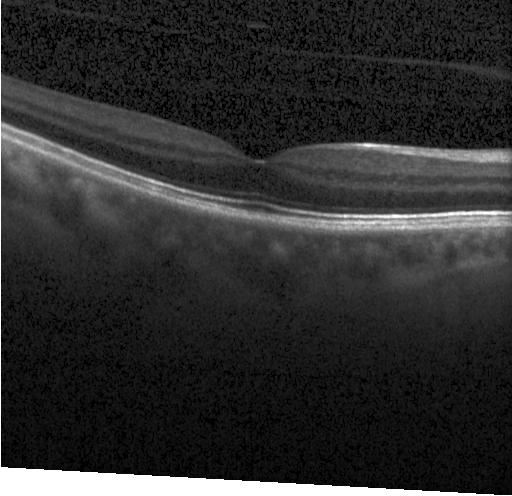 Retinal OCT B-scan — Diagnosis: no choroidal neovascularization, diabetic macular edema, or drusen.